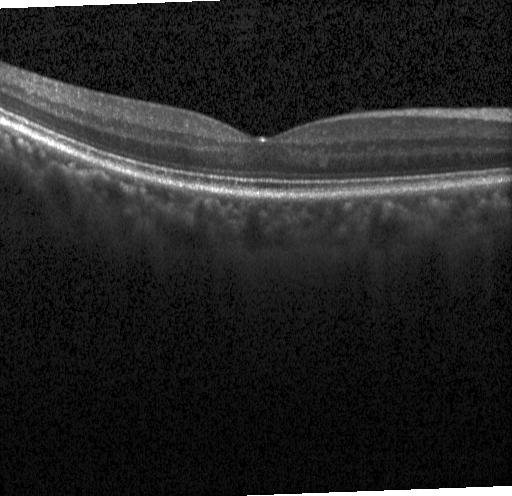
Optical coherence tomography scan. Dx: no evidence of CNV, DME, or drusen.